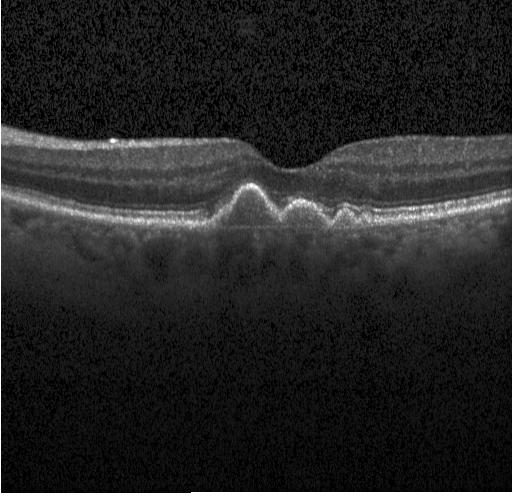 Optical coherence tomography scan. SD-OCT. Acquired on a Heidelberg Spectralis. Macular scan
Finding: multiple drusen.